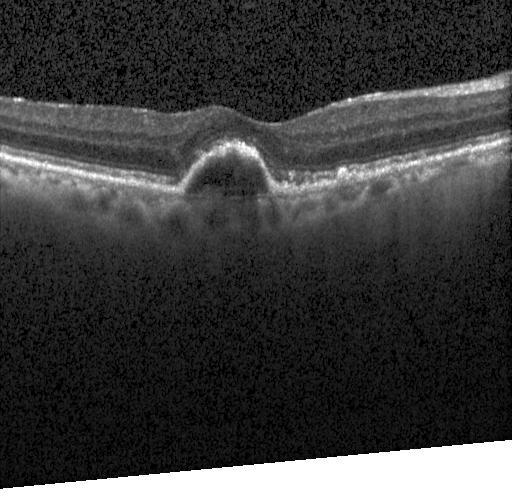
Horizontal scan through the fovea · optical coherence tomography B-scan.
A choroidal neovascular membrane.